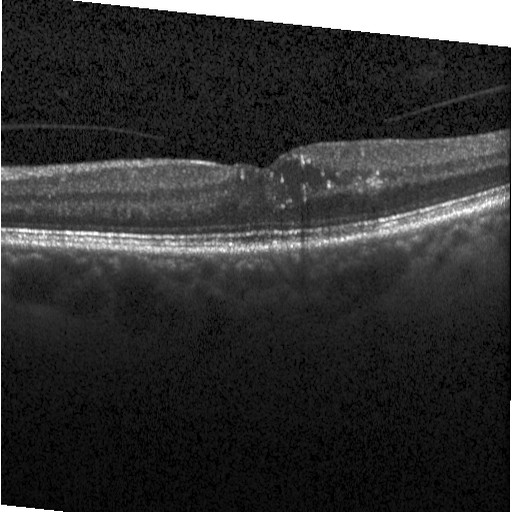
Diabetic macular edema (DME).